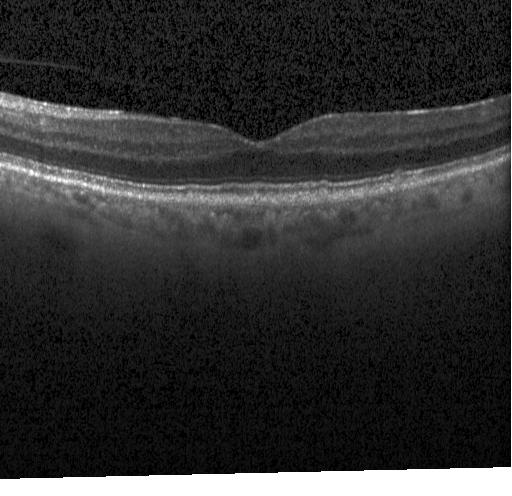
Macular OCT demonstrating sub-RPE drusenoid deposits.